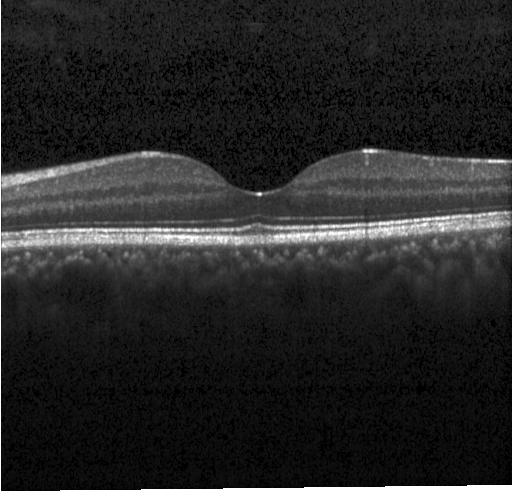 The scan shows neither choroidal neovascularization, diabetic macular edema, nor drusen.